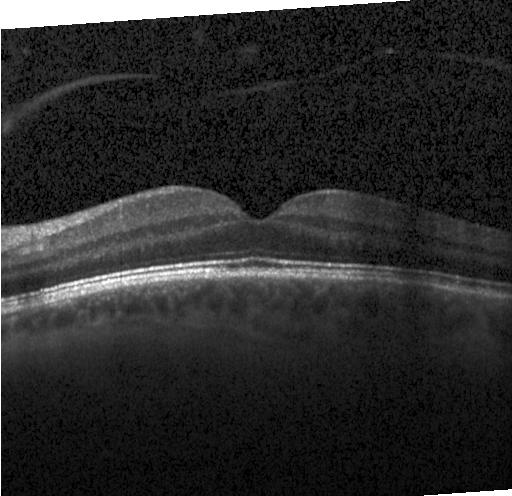

OCT finding: no evidence of choroidal neovascularization, diabetic macular edema, or drusen.